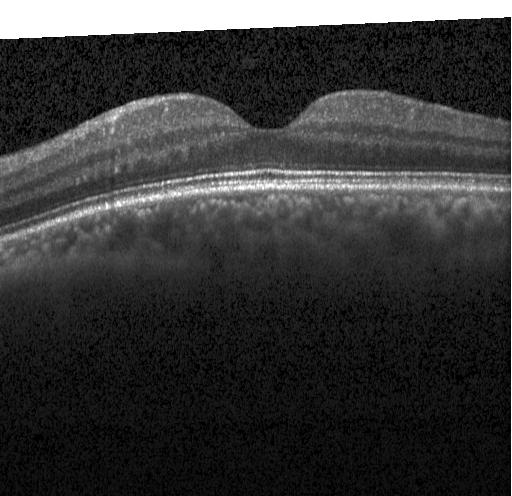
Retinal OCT B-scan. Spectral-domain OCT. Macular scan. Instrument: Heidelberg Spectralis — This B-scan demonstrates neither choroidal neovascularization, diabetic macular edema, nor drusen.